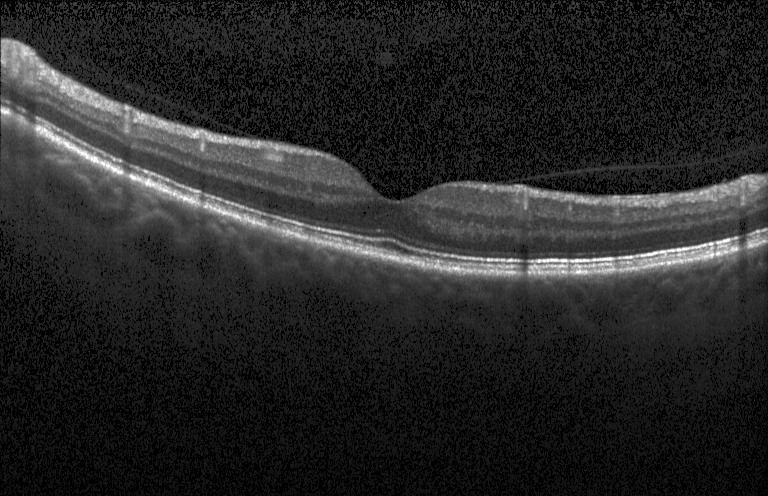 Macular OCT: no choroidal neovascularization, diabetic macular edema, or drusen.